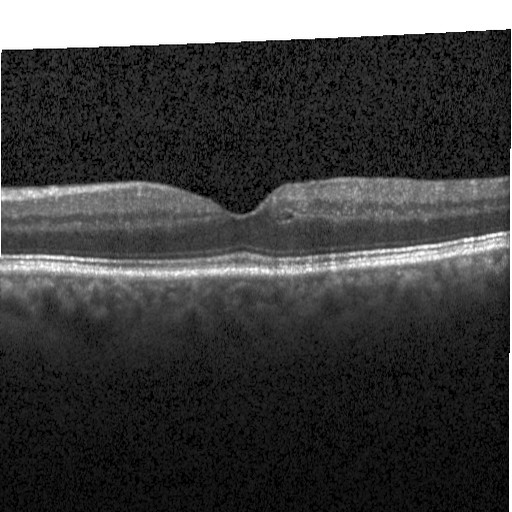
Retinal OCT cross-section
Dx: diabetic macular edema.